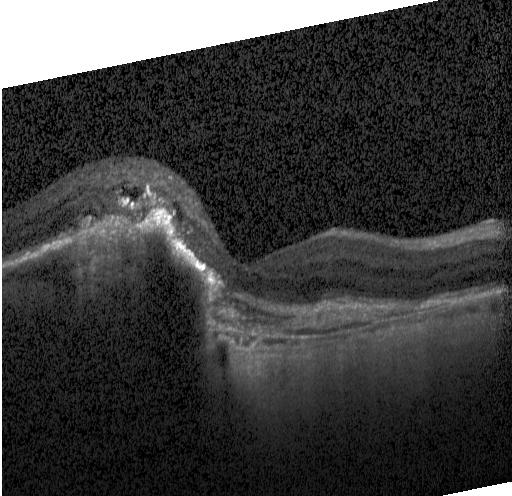

OCT B-scan
A choroidal neovascular membrane.